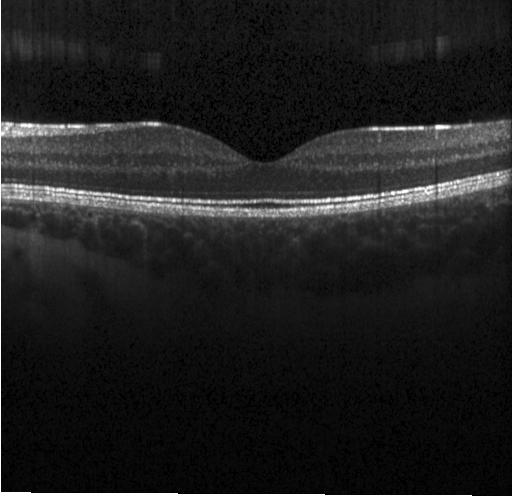 Retinal OCT B-scan
Dx: no choroidal neovascularization, no diabetic macular edema, and no drusen.